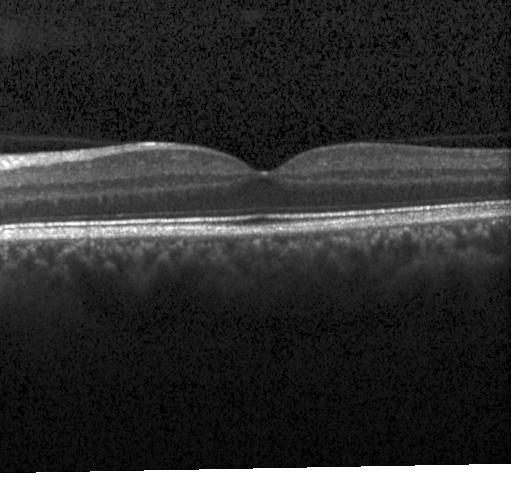

Spectral-domain optical coherence tomography, macular scan, optical coherence tomography B-scan, Heidelberg Spectralis
Impression: neither CNV, DME, nor drusen.